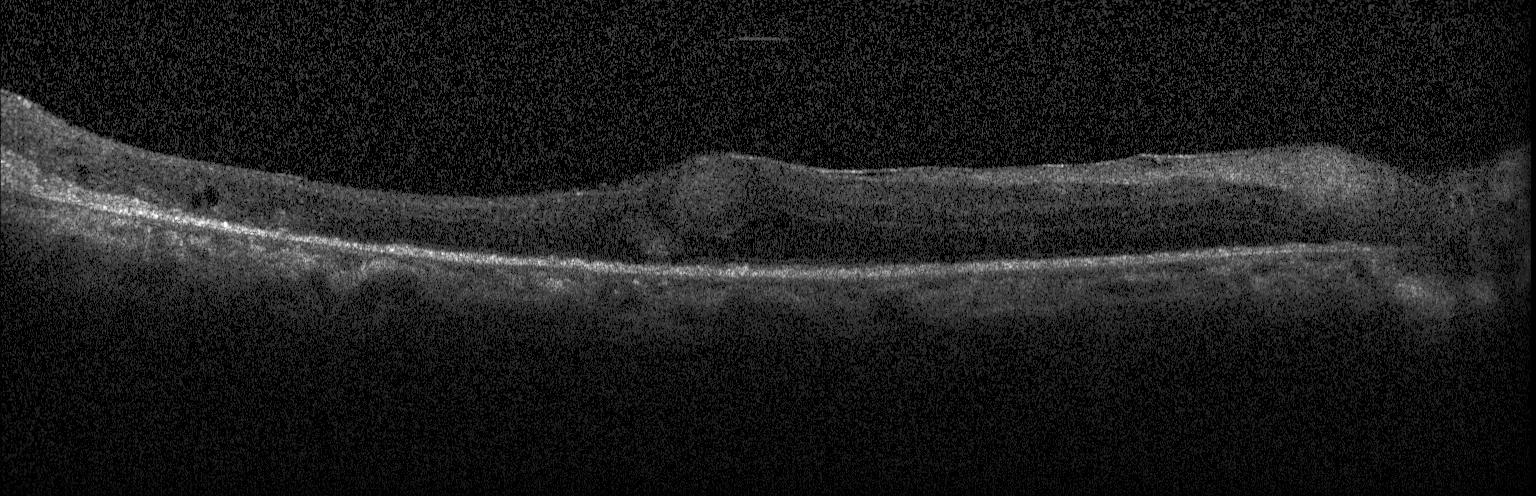
Diagnosis: diabetic macular edema (DME).